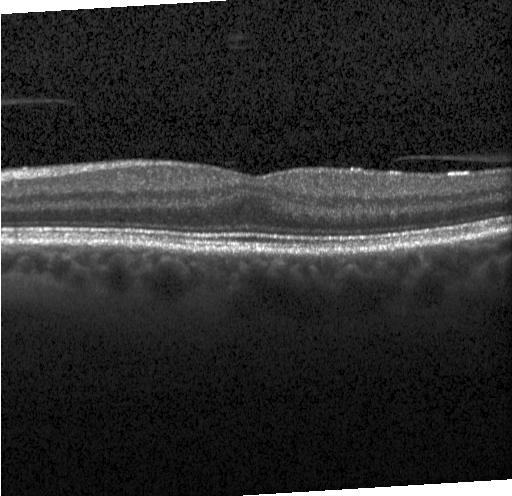 The scan shows neither CNV, DME, nor drusen.